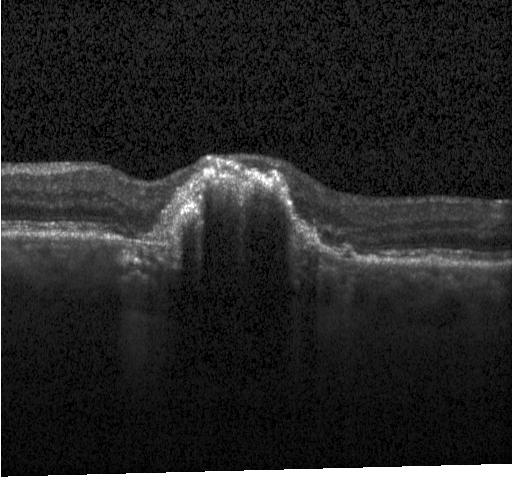
Spectral-domain OCT. Fovea-centered. OCT B-scan. Acquired on a Heidelberg Spectralis — Dx: a choroidal neovascular membrane.